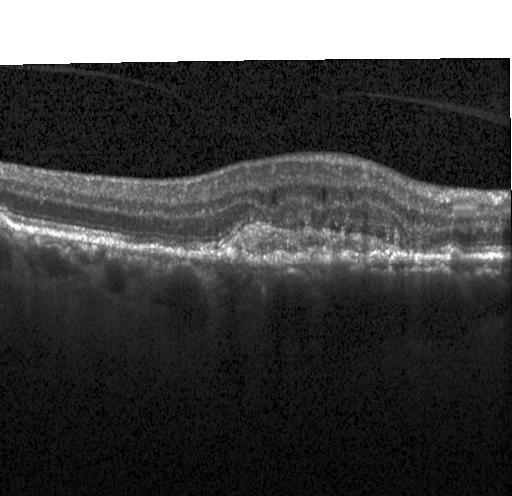 This B-scan demonstrates a choroidal neovascular membrane.